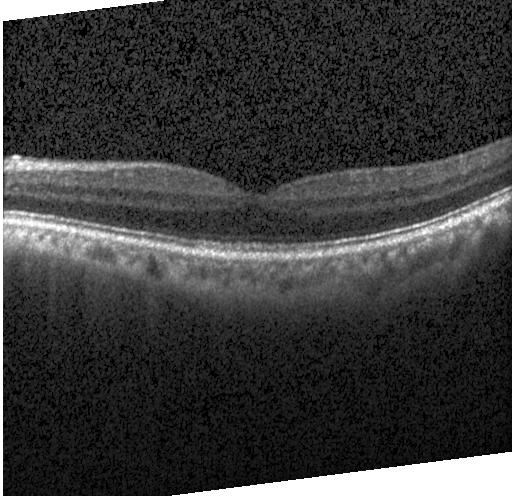 Fovea-centered, retinal OCT cross-section, spectral-domain OCT, Heidelberg Spectralis OCT system. Dx: neither choroidal neovascularization, diabetic macular edema, nor drusen.